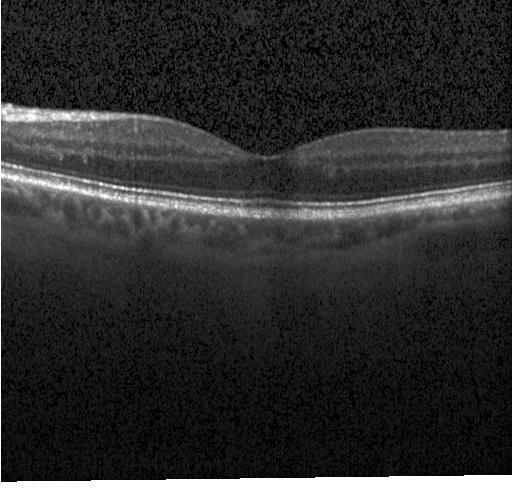 Spectral-domain OCT, OCT line scan, through the macula. The scan shows neither choroidal neovascularization, diabetic macular edema, nor drusen.